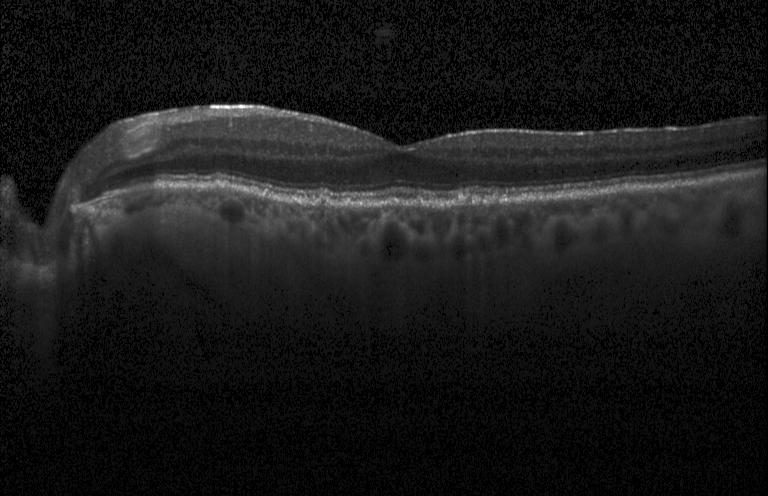
Heidelberg Spectralis OCT system, through the macula, retinal OCT cross-section. Multiple drusen.